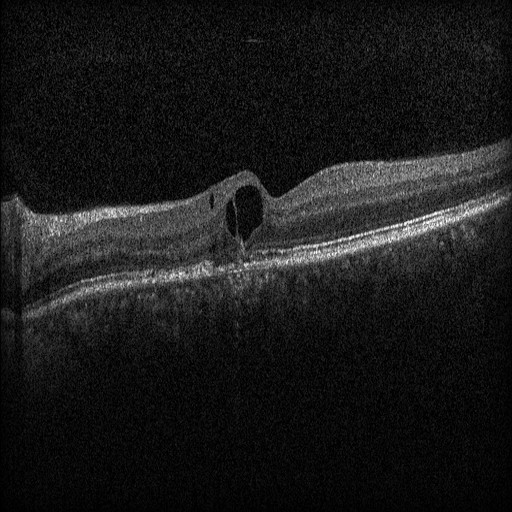
OCT line scan; spectral-domain optical coherence tomography; instrument: Heidelberg Spectralis; through the macula — Dx: diabetic macular edema.